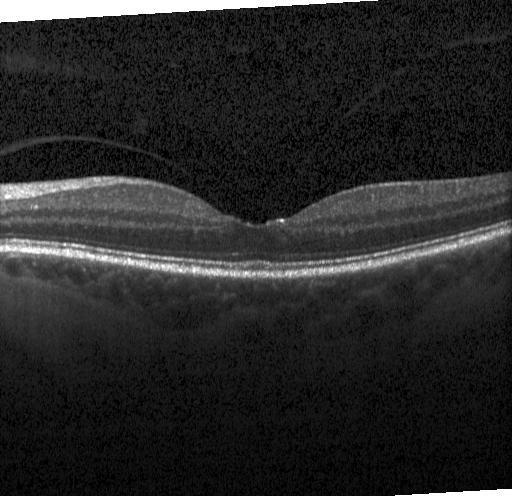

SD-OCT · through the macula · OCT B-scan.
Diagnosis: no choroidal neovascularization, no diabetic macular edema, and no drusen.